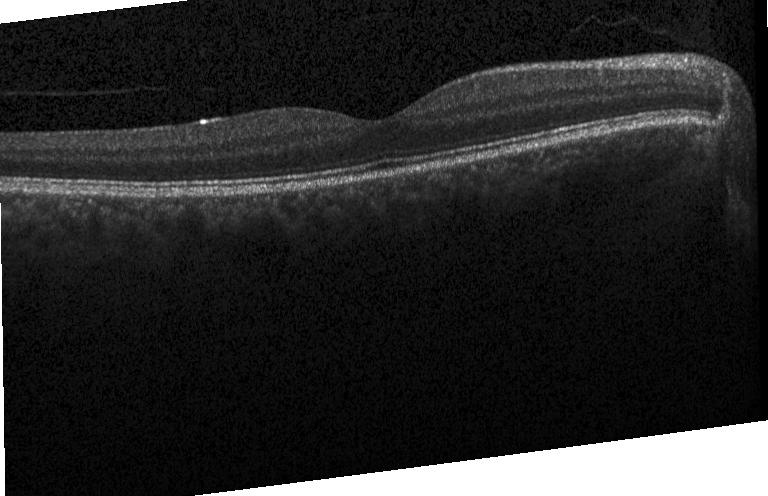
OCT B-scan showing no evidence of CNV, DME, or drusen.